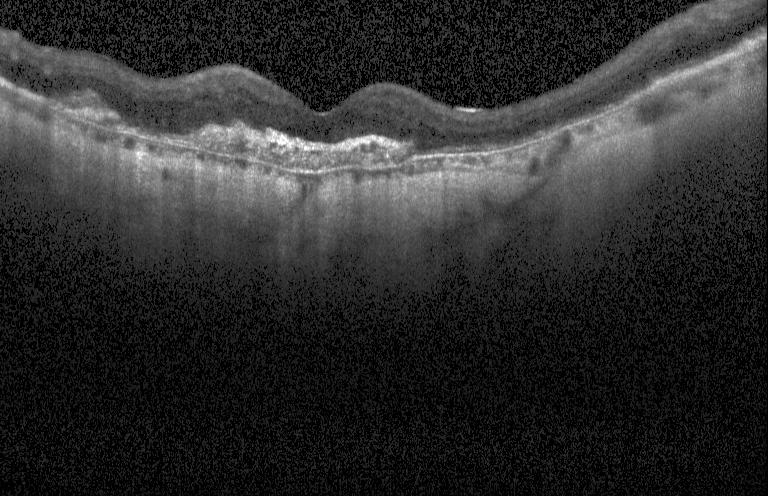
Spectral-domain OCT B-scan: CNV.